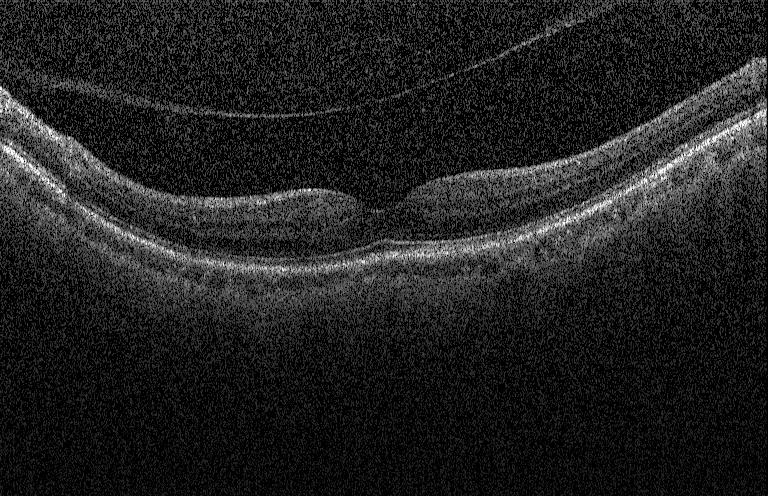 Impression: no choroidal neovascularization, diabetic macular edema, or drusen.